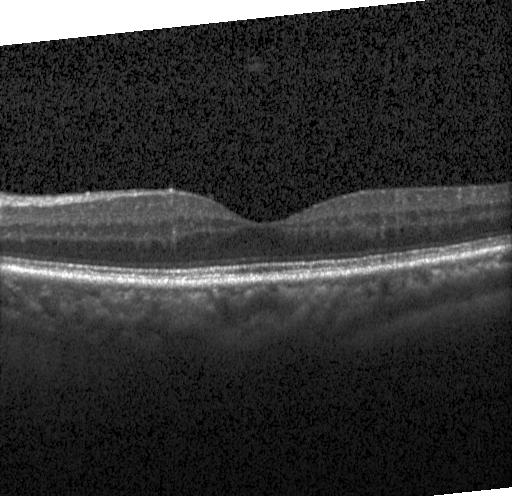

Retinal OCT cross-section. Through the macula. Impression: no choroidal neovascularization, diabetic macular edema, or drusen.